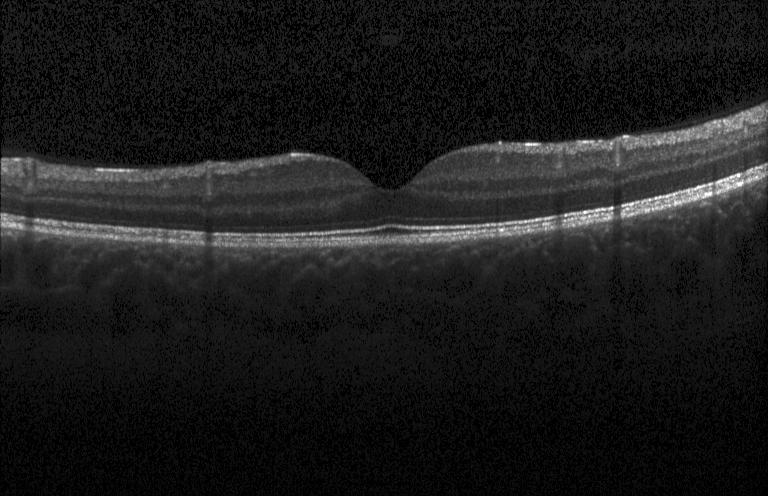 Spectral-domain OCT. Retinal OCT B-scan. Heidelberg Spectralis OCT system. Centered on the fovea
Macular OCT: no evidence of CNV, DME, or drusen.